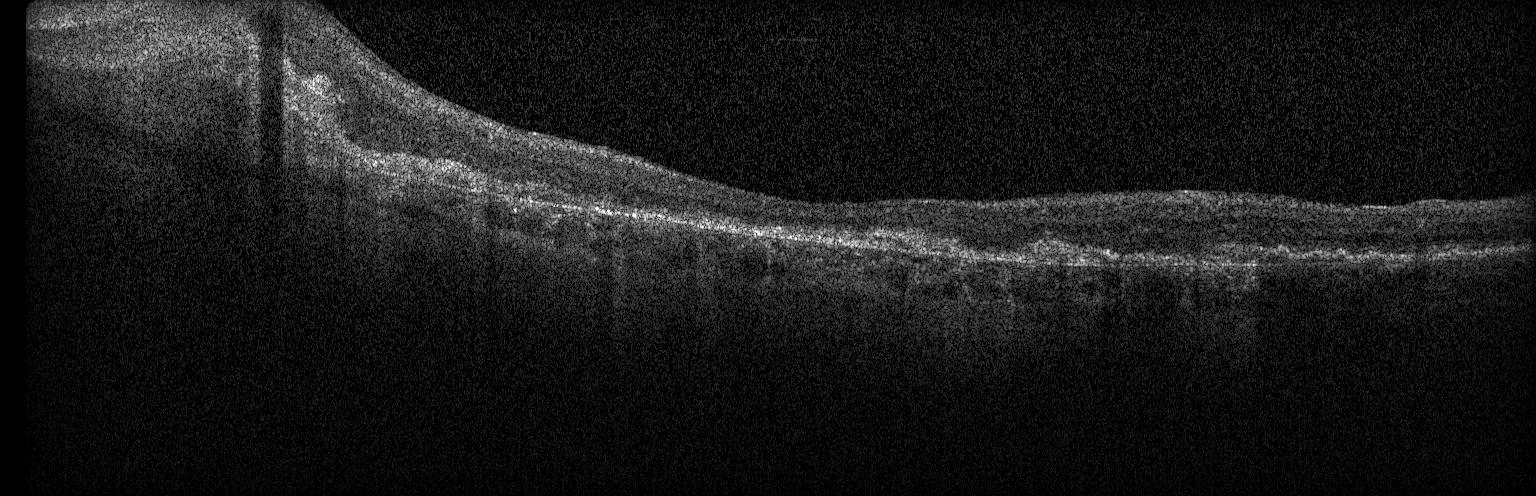
Optical coherence tomography scan; Heidelberg Spectralis OCT system; fovea-centered; SD-OCT. Assessment: choroidal neovascularization.